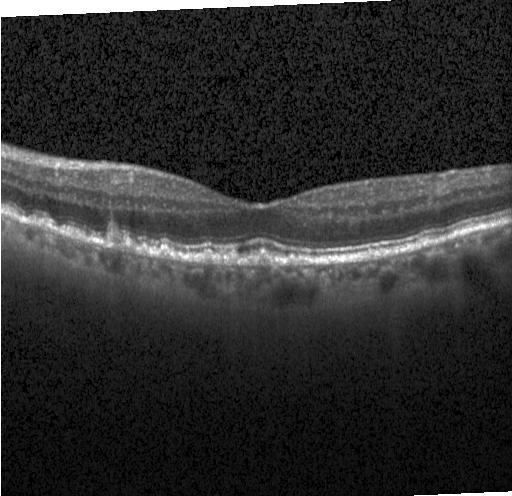 Instrument: Heidelberg Spectralis, SD-OCT, fovea-centered, optical coherence tomography scan
Dx: drusen.